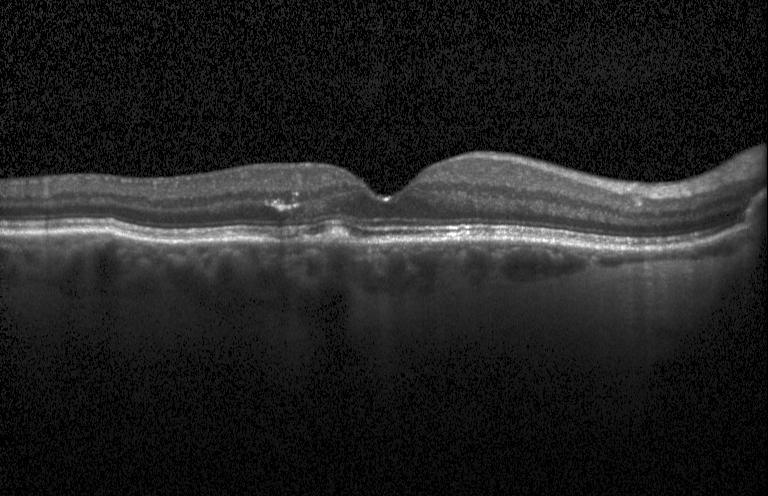 Horizontal scan through the fovea, OCT B-scan, instrument: Heidelberg Spectralis.
Dx: multiple drusen.